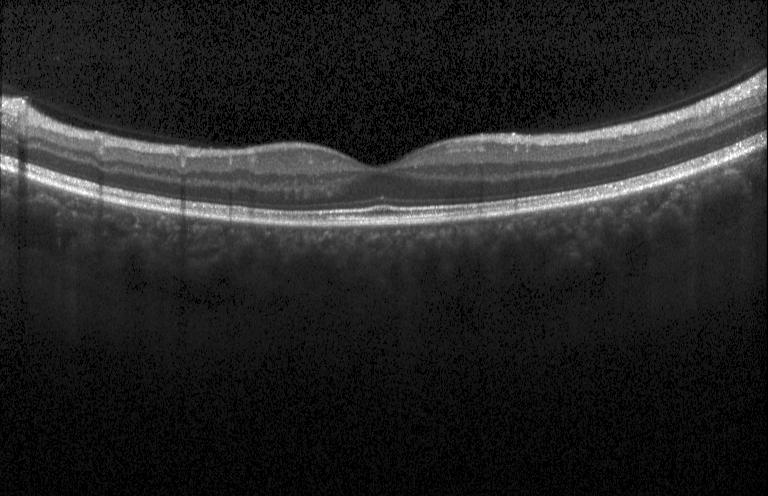 OCT line scan. Finding: no CNV, DME, or drusen.